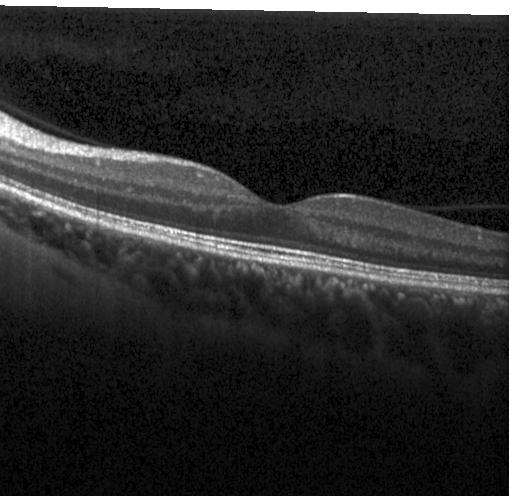

OCT finding: no CNV, no DME, and no drusen.